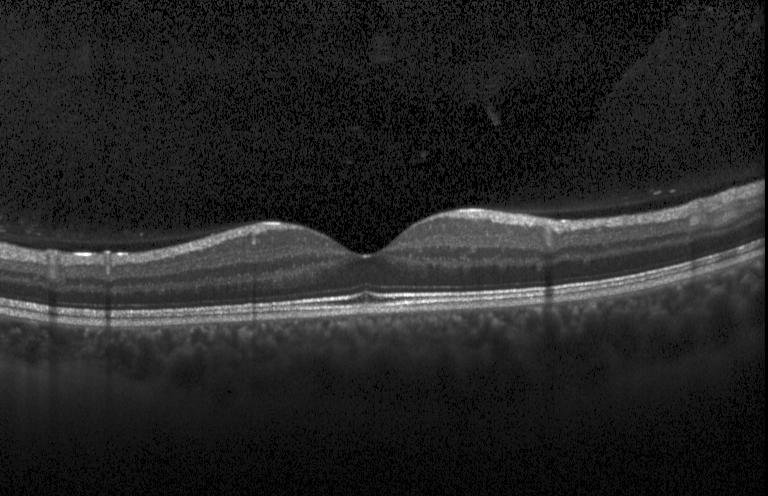

Impression: no choroidal neovascularization, diabetic macular edema, or drusen.